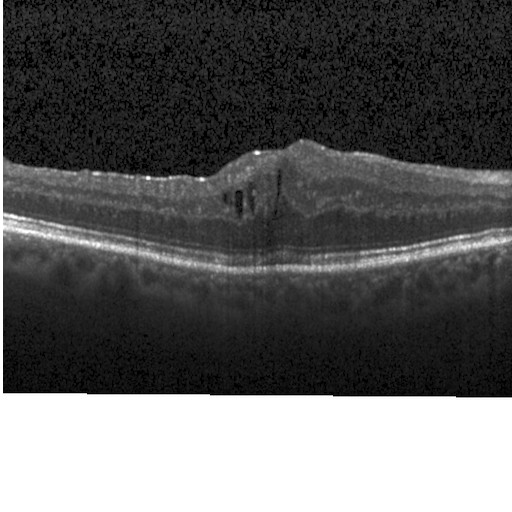

Retinal OCT cross-section showing DME.